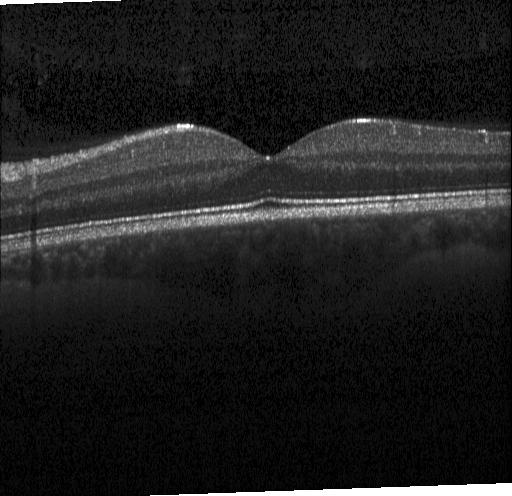

Assessment: no CNV, DME, or drusen.